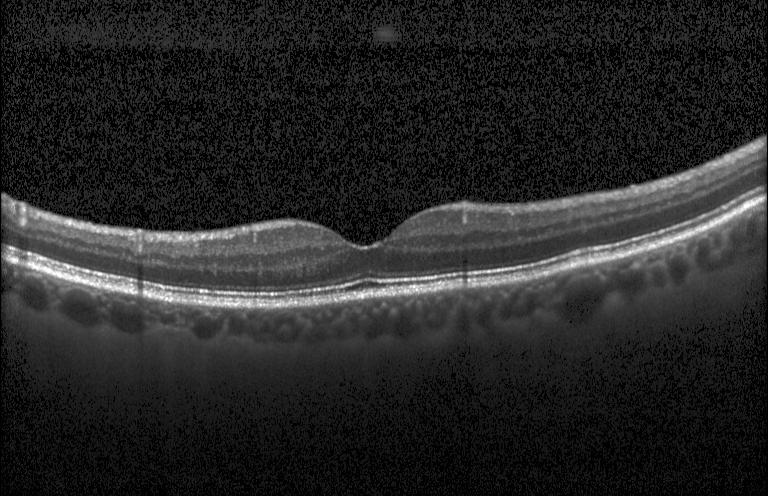

OCT B-scan
Impression: no CNV, DME, or drusen.